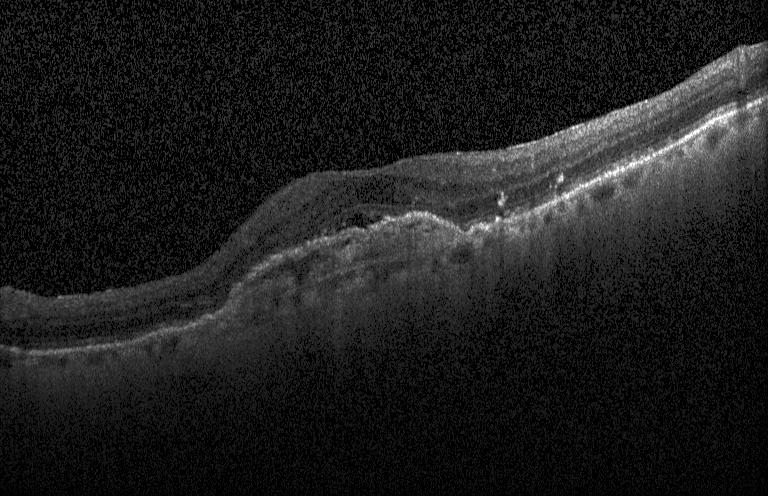
Optical coherence tomography B-scan · SD-OCT · fovea-centered
The scan shows a choroidal neovascular membrane.